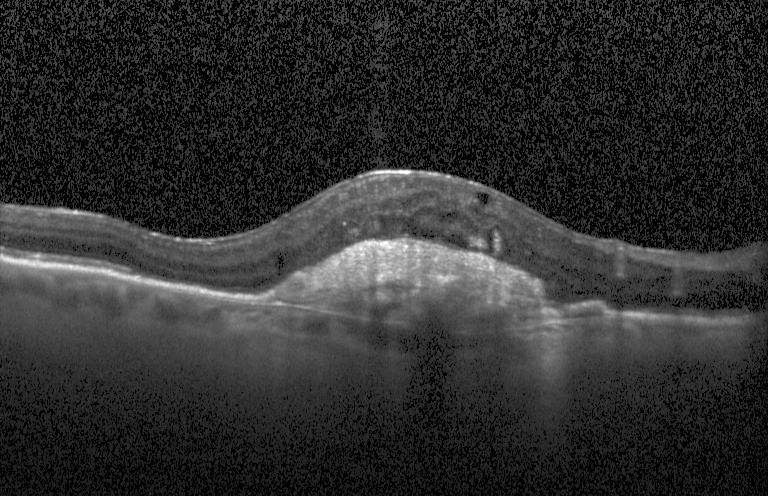 Retinal OCT cross-section — This B-scan demonstrates choroidal neovascularization.